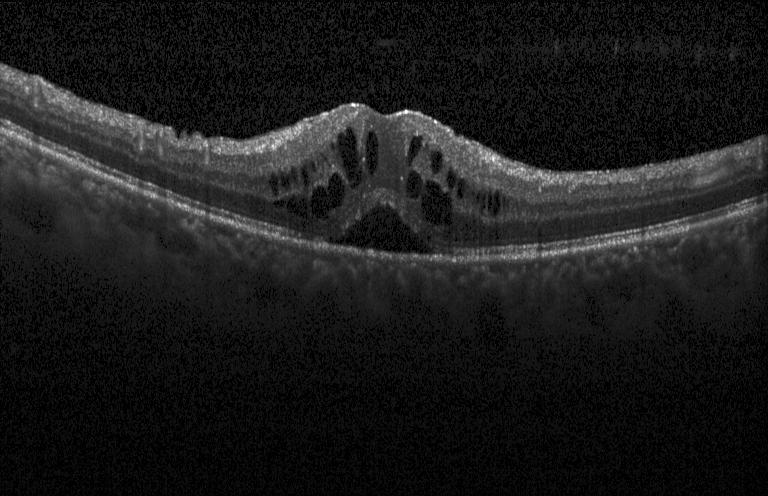

Macular OCT demonstrating diabetic macular edema.